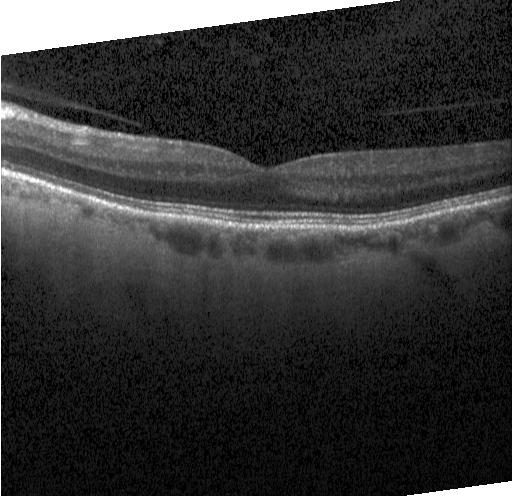 OCT line scan. Spectral-domain optical coherence tomography.
Diagnosis: no CNV, no DME, and no drusen.